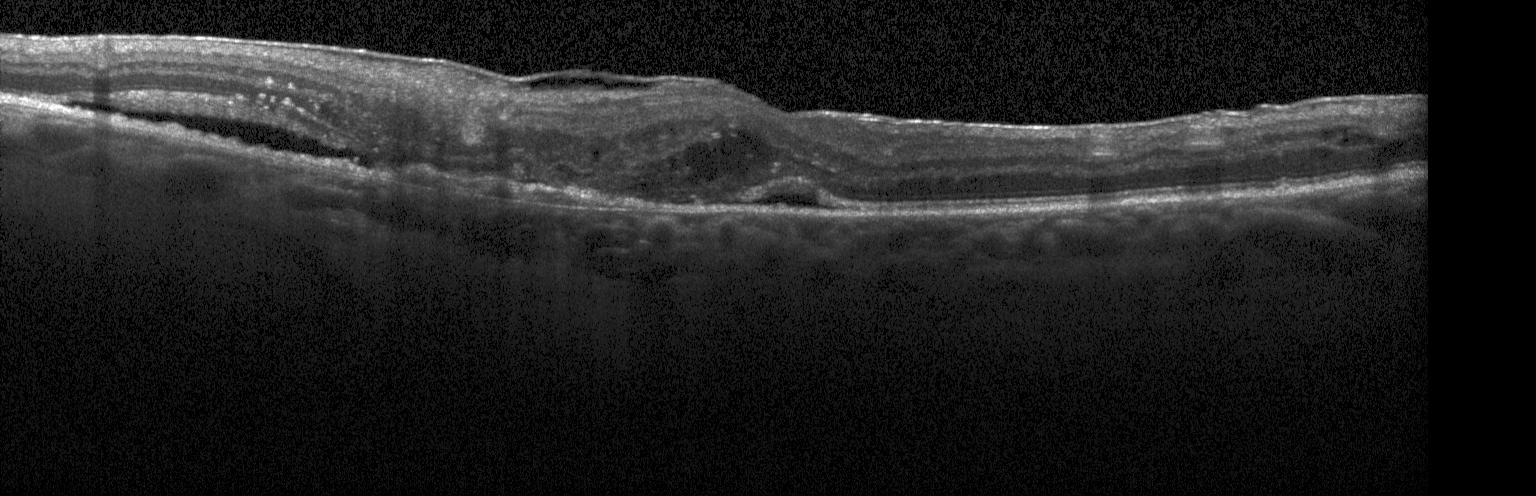 Retinal OCT B-scan, spectral-domain OCT
Impression: choroidal neovascularization (CNV).